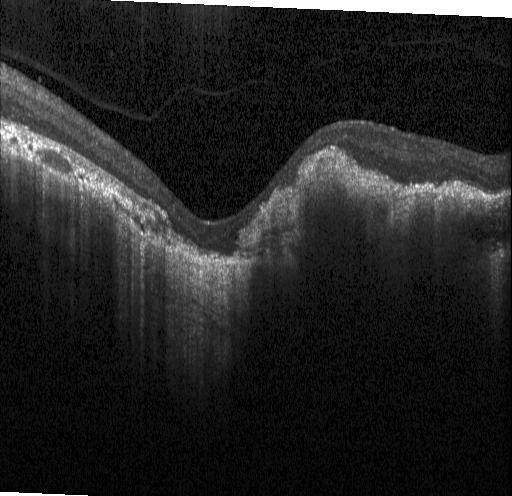
Impression: choroidal neovascularization (CNV).